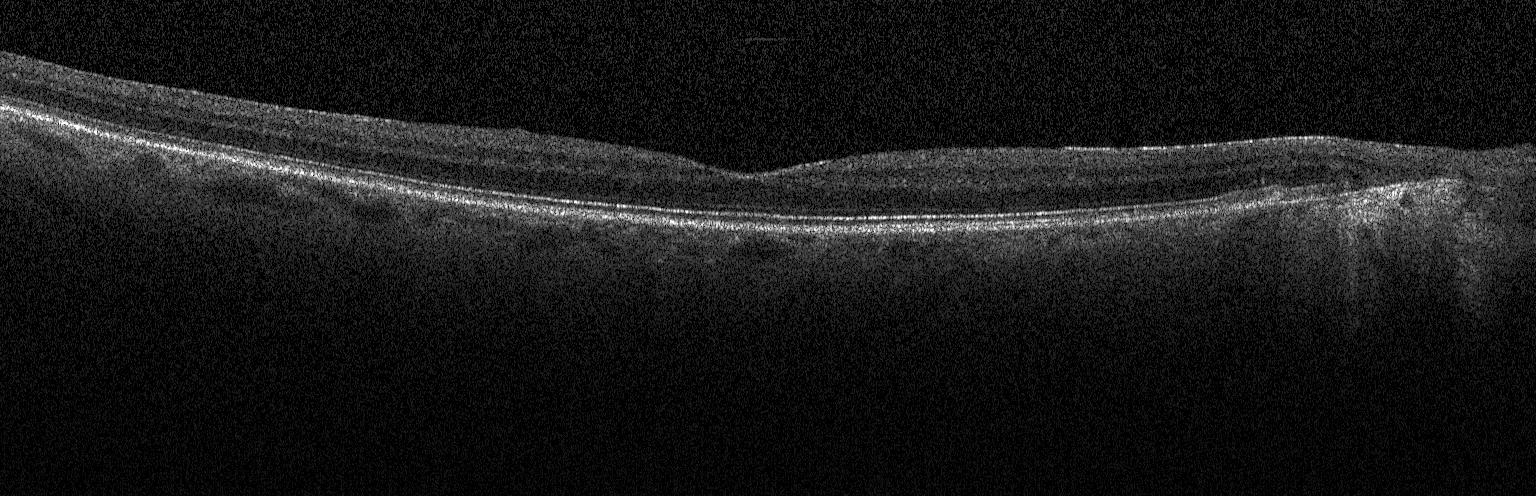
Diagnosis: neither choroidal neovascularization, diabetic macular edema, nor drusen.